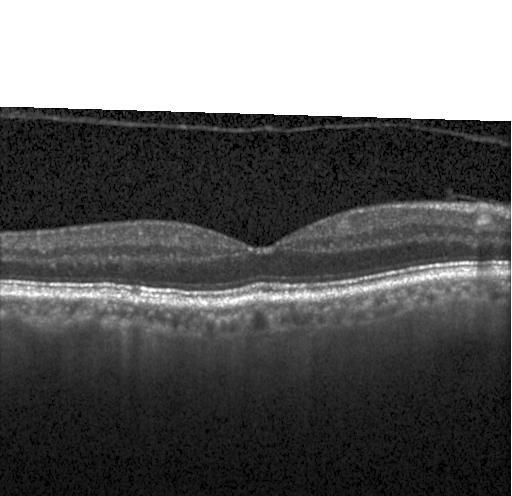
Finding: no evidence of CNV, DME, or drusen.